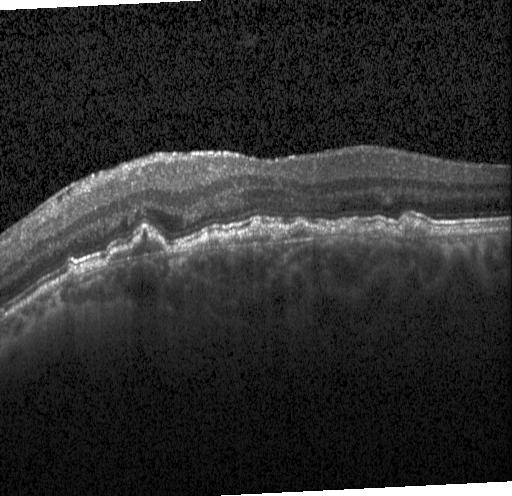 Retinal OCT cross-section. Impression: a choroidal neovascular membrane.